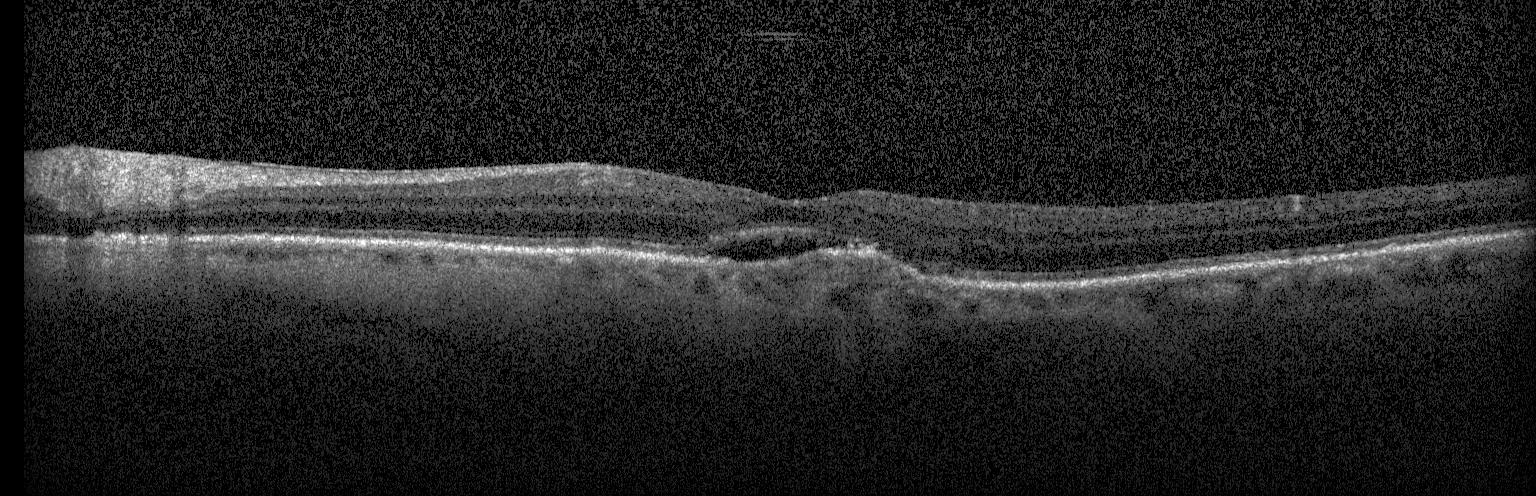
Assessment: a choroidal neovascular membrane.